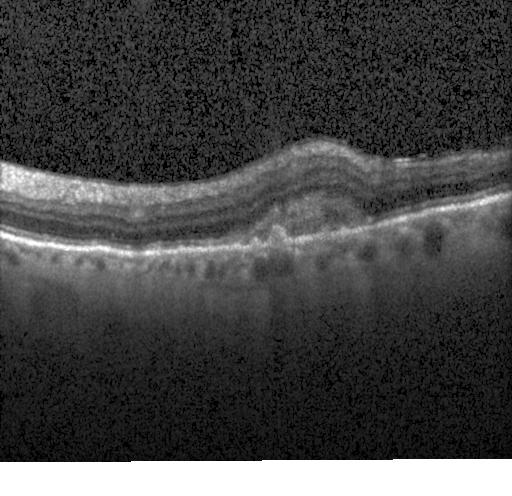
Spectral-domain OCT B-scan: CNV.